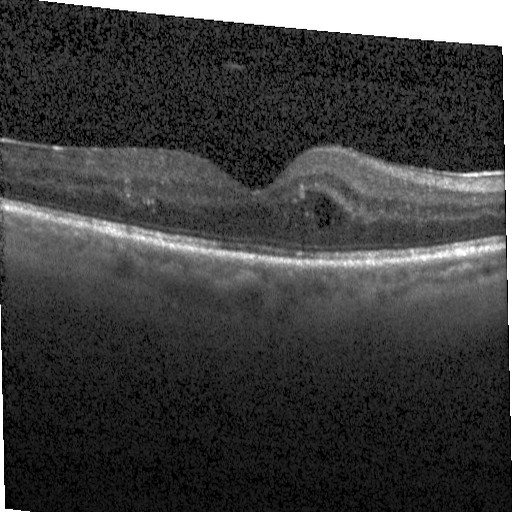
Retinal OCT B-scan. Instrument: Heidelberg Spectralis. This B-scan demonstrates diabetic macular edema.